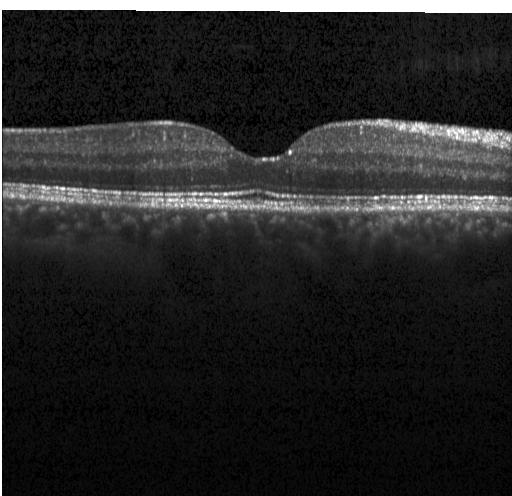

Optical coherence tomography B-scan · Heidelberg Spectralis OCT system. Diagnosis: no evidence of choroidal neovascularization, diabetic macular edema, or drusen.